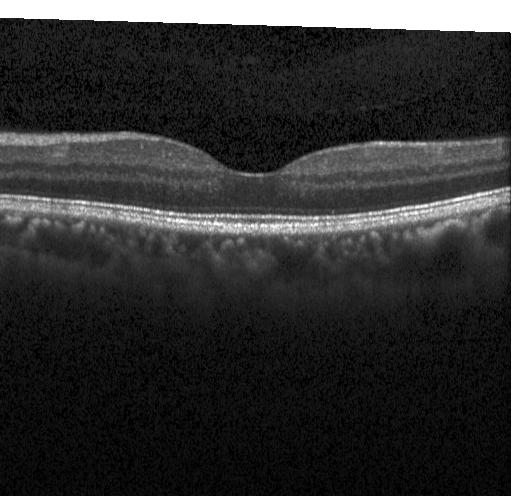 Diagnosis: no choroidal neovascularization, diabetic macular edema, or drusen.